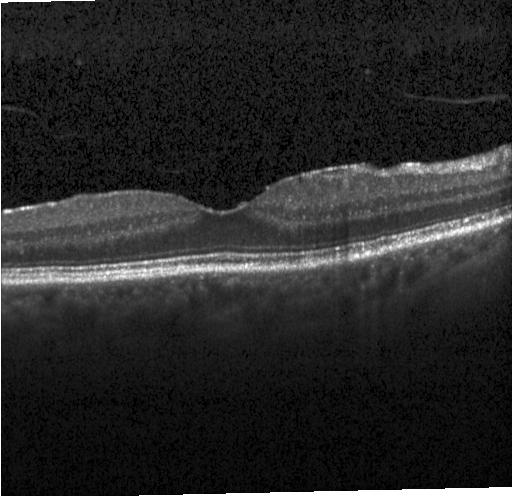

Optical coherence tomography B-scan — Assessment: no choroidal neovascularization, diabetic macular edema, or drusen.